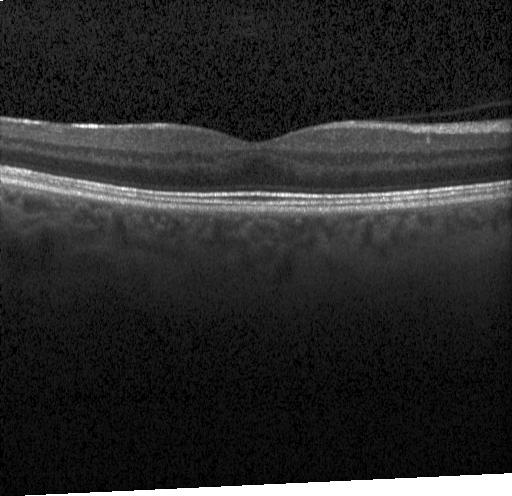 Impression: no choroidal neovascularization, diabetic macular edema, or drusen.